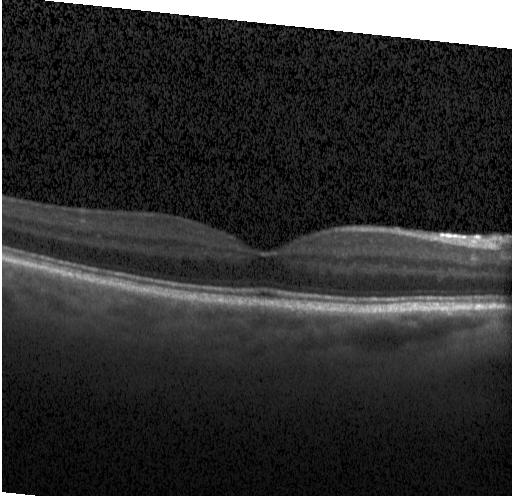
Diagnosis: no choroidal neovascularization, diabetic macular edema, or drusen.